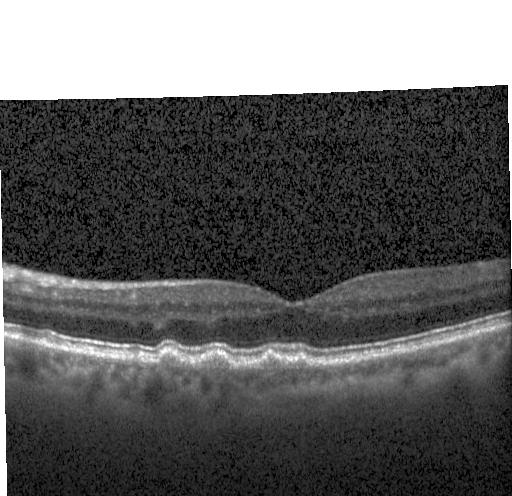
Assessment: sub-RPE drusenoid deposits.